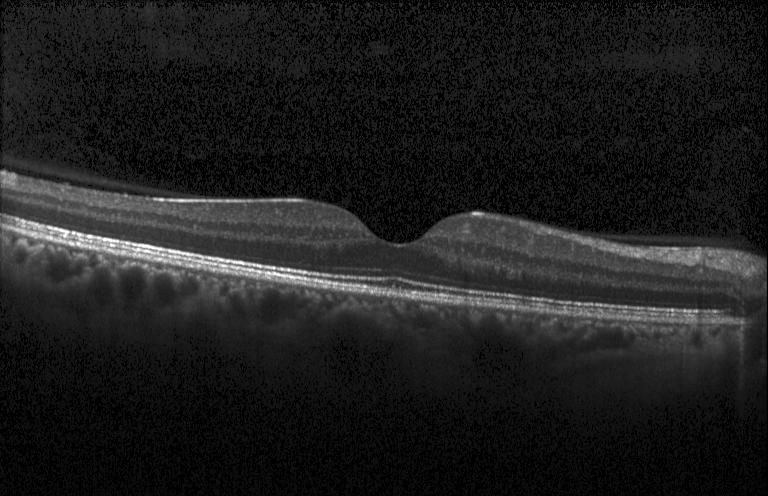

Fovea-centered; optical coherence tomography B-scan; spectral-domain OCT. The scan shows no evidence of CNV, DME, or drusen.